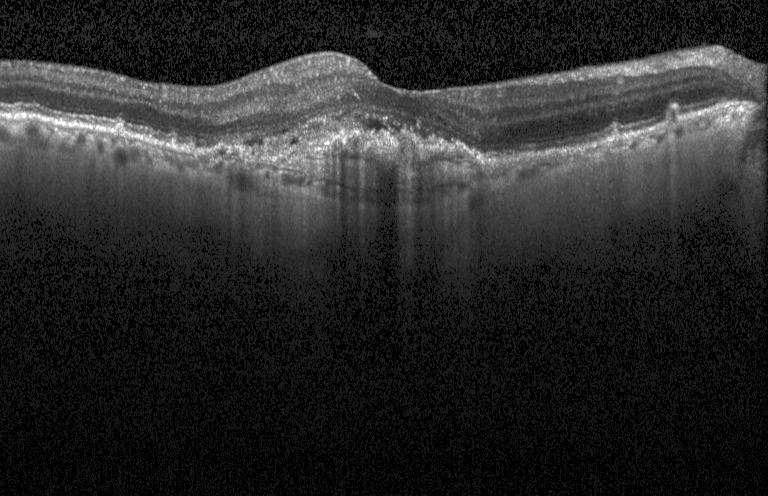 Spectral-domain OCT; optical coherence tomography scan; acquired on a Heidelberg Spectralis. Diagnosis: a choroidal neovascular membrane.